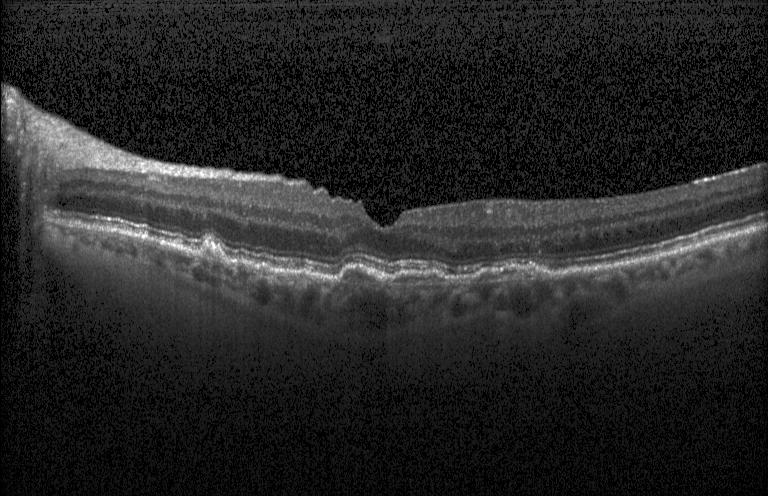
Macular OCT demonstrating sub-RPE drusenoid deposits.